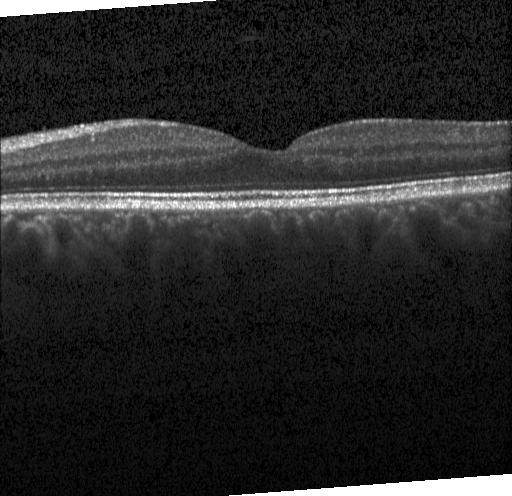
Heidelberg Spectralis OCT system. Macular scan. Retinal OCT B-scan
Dx: no evidence of CNV, DME, or drusen.